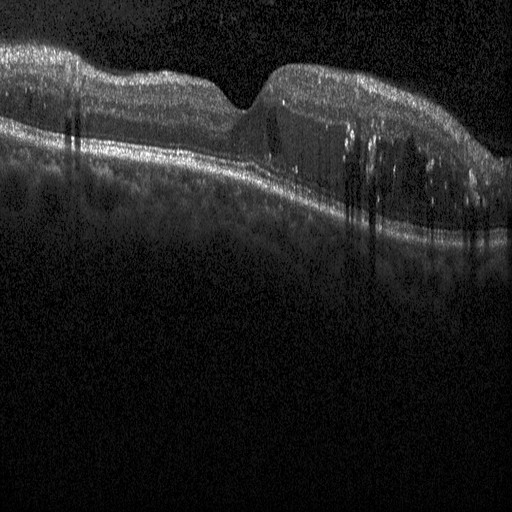
OCT line scan. Finding: diabetic macular edema (DME).